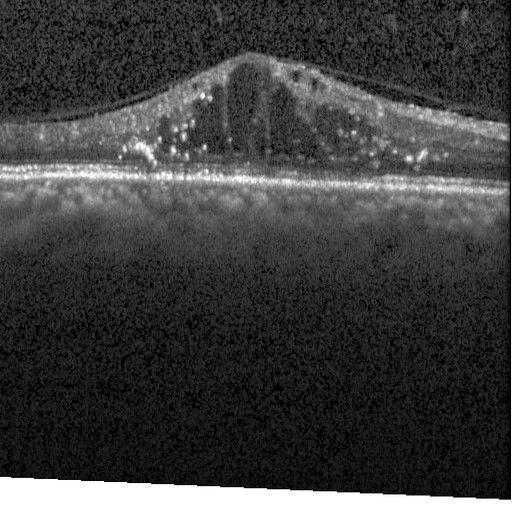

Acquired on a Heidelberg Spectralis; spectral-domain OCT; horizontal scan through the fovea; optical coherence tomography scan — Diabetic macular edema.